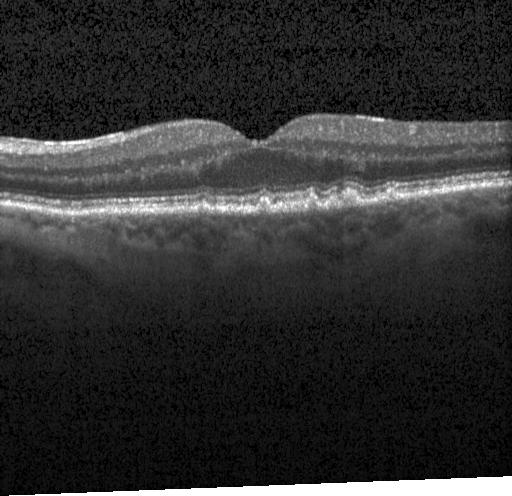

OCT B-scan.
Assessment: drusen.